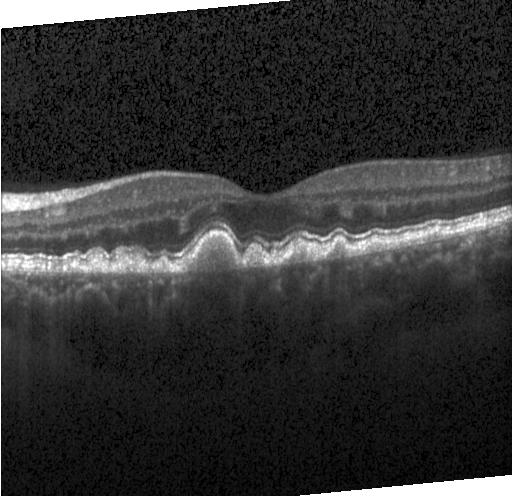 Retinal OCT cross-section; centered on the fovea; instrument: Heidelberg Spectralis; SD-OCT
Drusen.